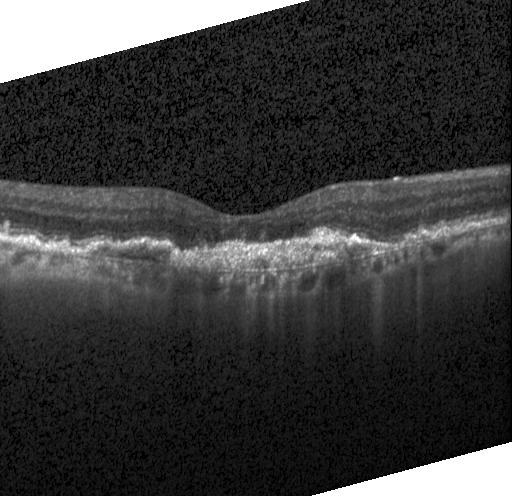 Through the macula, retinal OCT B-scan, Heidelberg Spectralis OCT system, spectral-domain optical coherence tomography. Finding: a choroidal neovascular membrane.